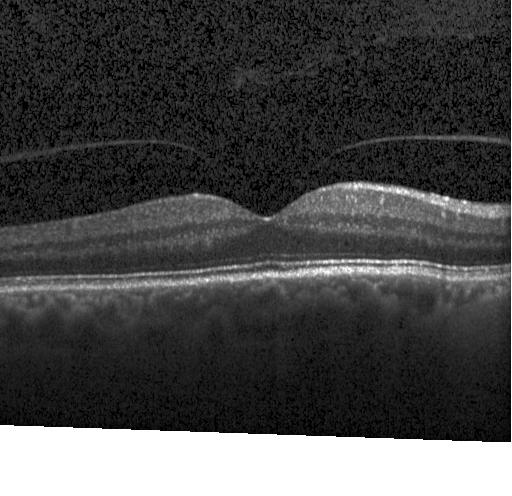 OCT scan showing neither choroidal neovascularization, diabetic macular edema, nor drusen.